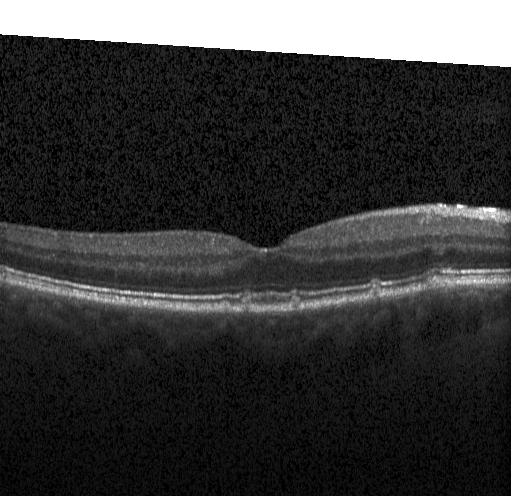

Retinal OCT cross-section · SD-OCT — Assessment: sub-RPE drusenoid deposits.